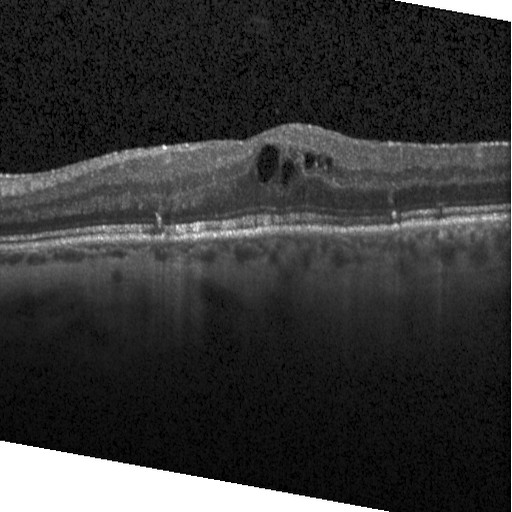 Acquired on a Heidelberg Spectralis, retinal OCT B-scan. Diagnosis: diabetic macular edema (DME).